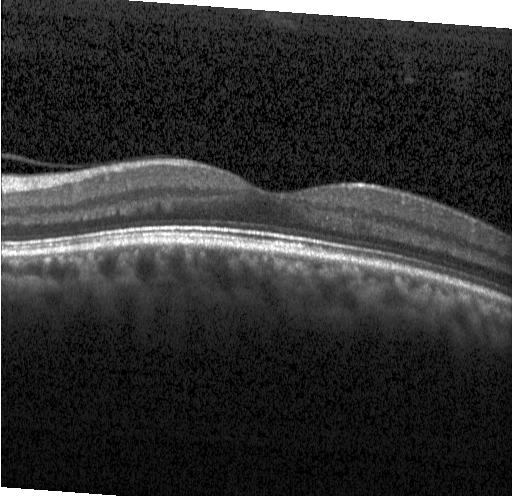 Optical coherence tomography scan.
Assessment: neither CNV, DME, nor drusen.